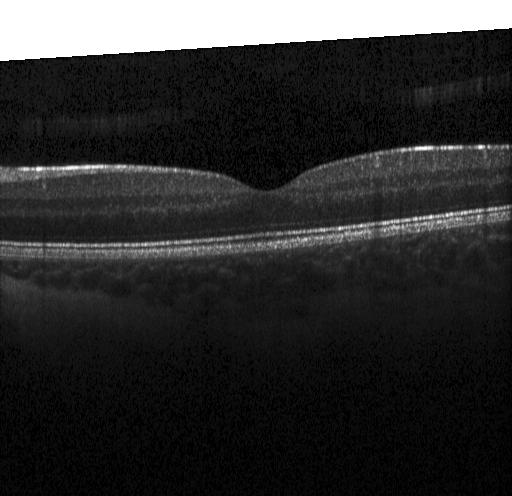

Impression: no CNV, DME, or drusen.